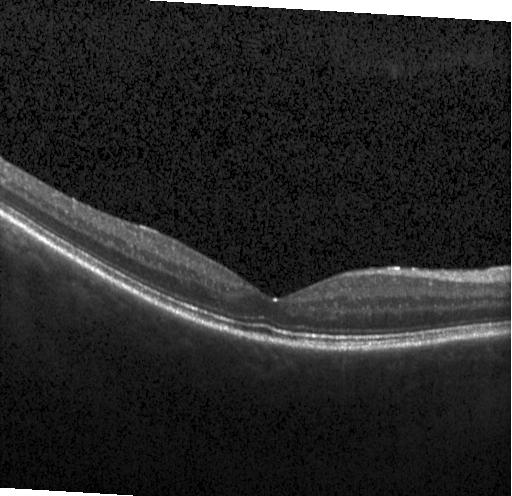

Assessment: no CNV, no DME, and no drusen.